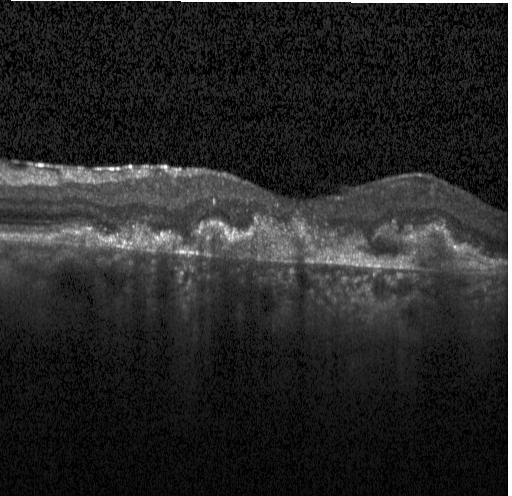

Retinal OCT cross-section, acquired on a Heidelberg Spectralis.
Diagnosis: CNV.